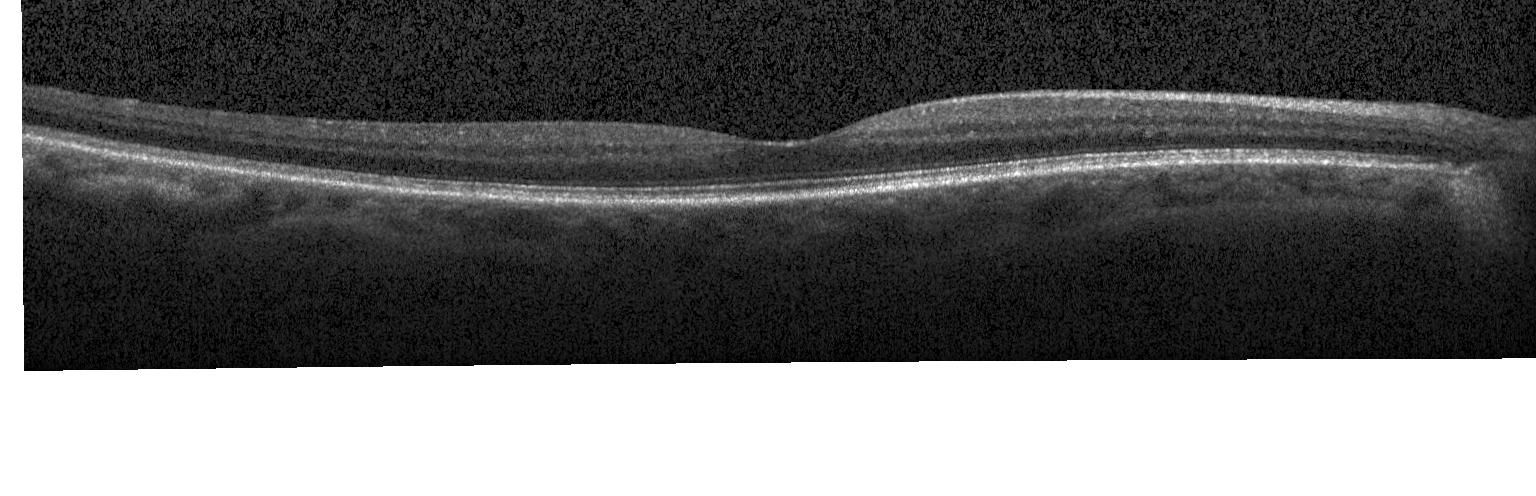 OCT B-scan. Dx: no choroidal neovascularization, diabetic macular edema, or drusen.